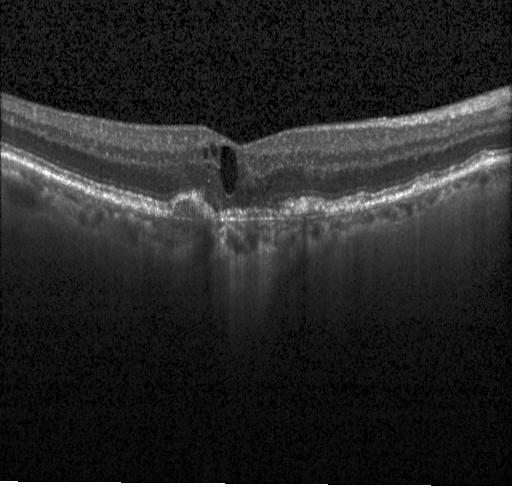 OCT B-scan · macular scan · instrument: Heidelberg Spectralis · SD-OCT.
Diagnosis: a choroidal neovascular membrane.